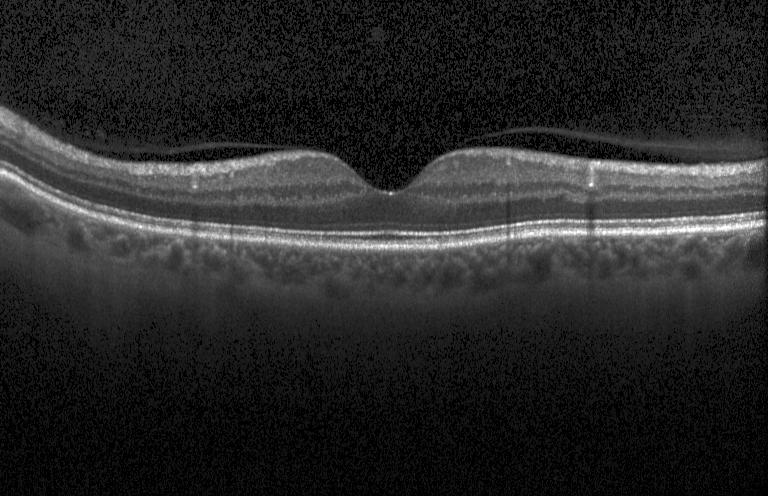
SD-OCT; OCT line scan; Heidelberg Spectralis OCT system
No choroidal neovascularization, diabetic macular edema, or drusen.